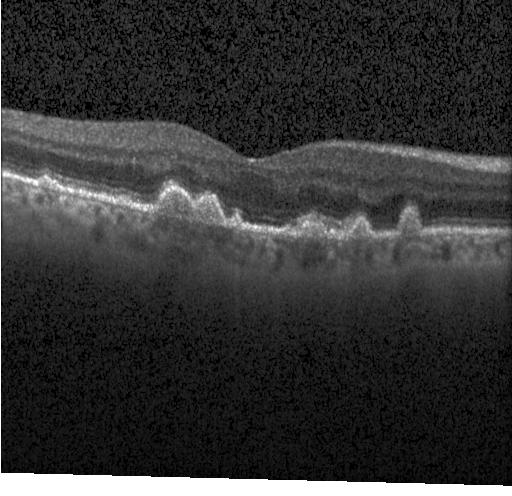

Retinal OCT B-scan, spectral-domain OCT.
Finding: sub-RPE drusenoid deposits.